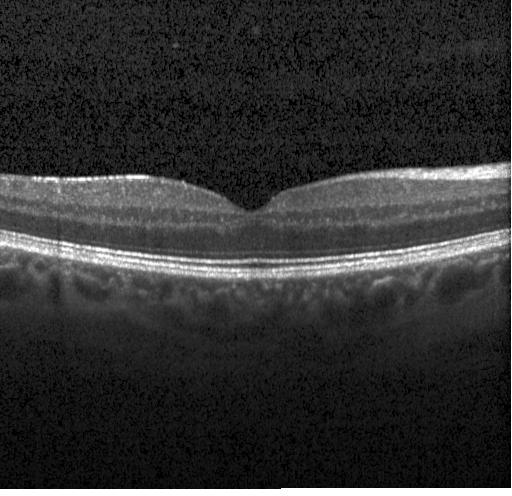 Dx: neither choroidal neovascularization, diabetic macular edema, nor drusen.